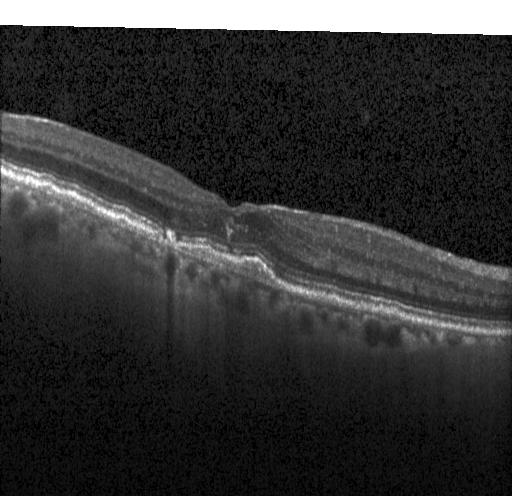
Impression: choroidal neovascularization.